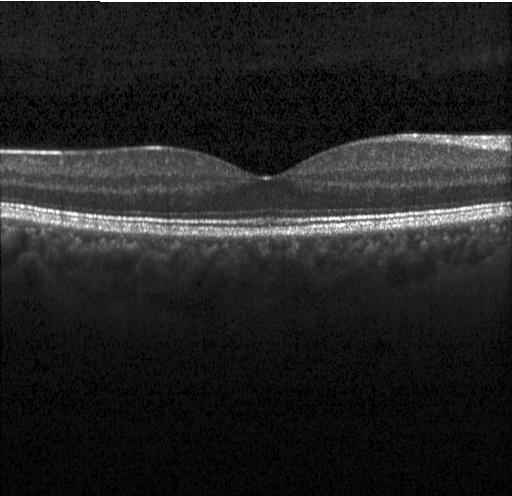 Instrument: Heidelberg Spectralis. Optical coherence tomography B-scan
No evidence of CNV, DME, or drusen.